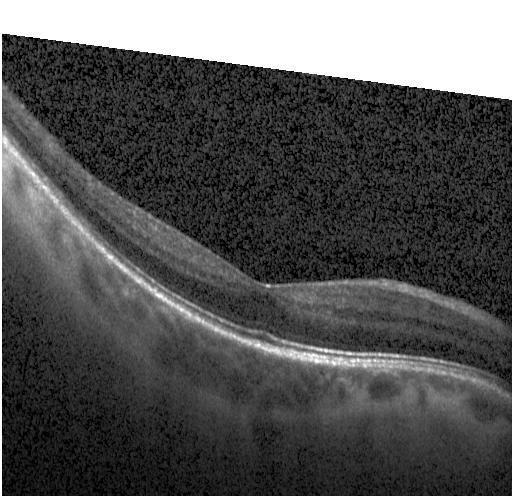
Optical coherence tomography B-scan. Spectral-domain OCT. This B-scan demonstrates neither choroidal neovascularization, diabetic macular edema, nor drusen.